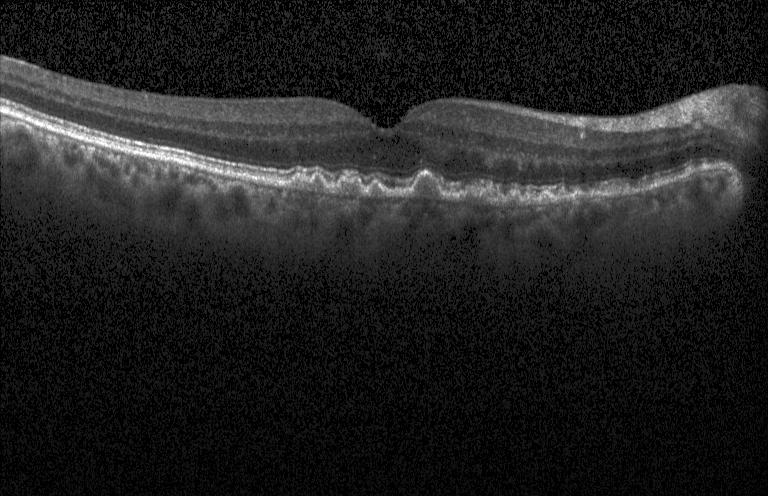 Spectral-domain OCT; retinal OCT cross-section. The scan shows sub-RPE drusenoid deposits.